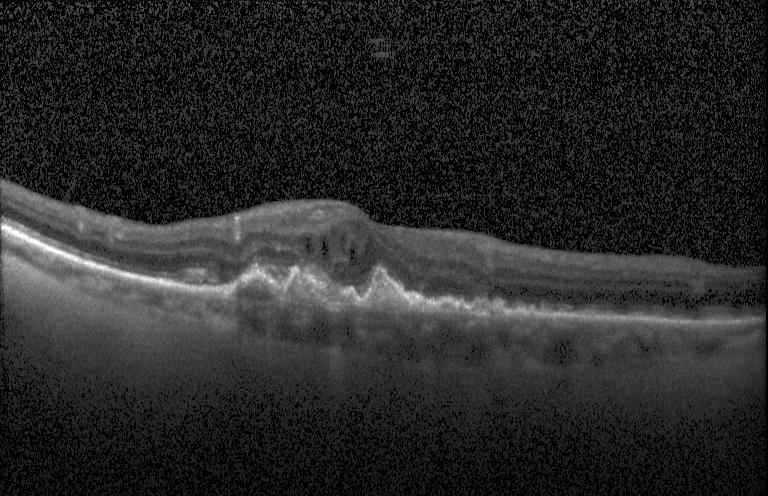

Heidelberg Spectralis OCT system, optical coherence tomography scan — Finding: CNV.